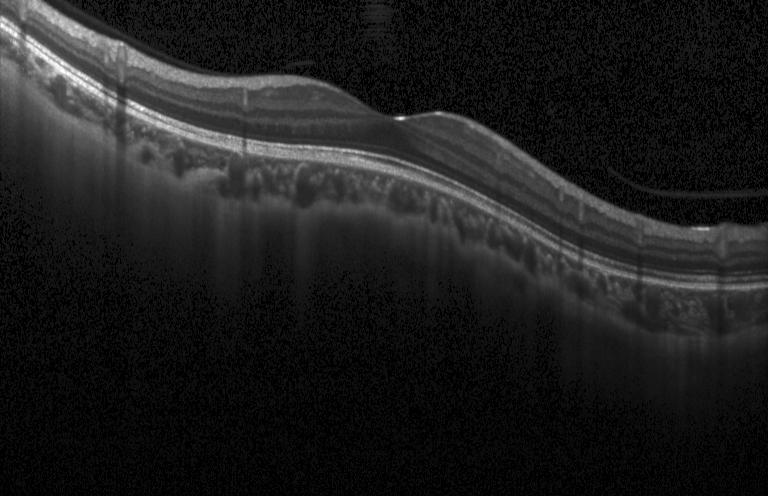

Fovea-centered; spectral-domain OCT; Heidelberg Spectralis; retinal OCT cross-section.
Impression: no CNV, DME, or drusen.